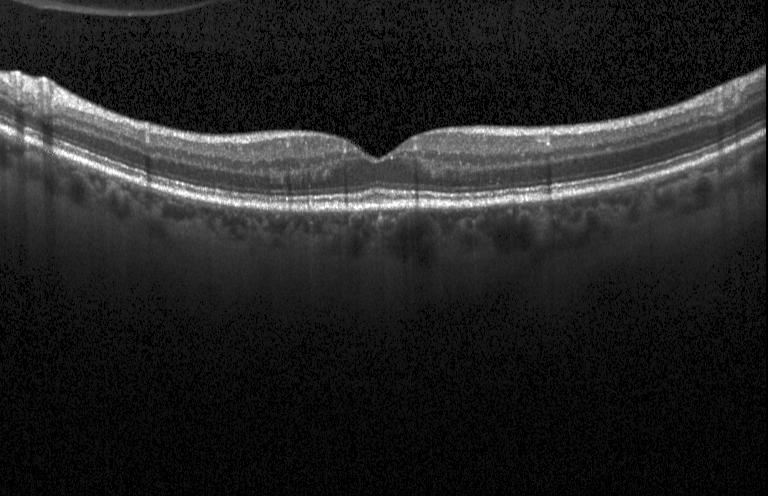 OCT B-scan, centered on the fovea, instrument: Heidelberg Spectralis — OCT finding: neither CNV, DME, nor drusen.